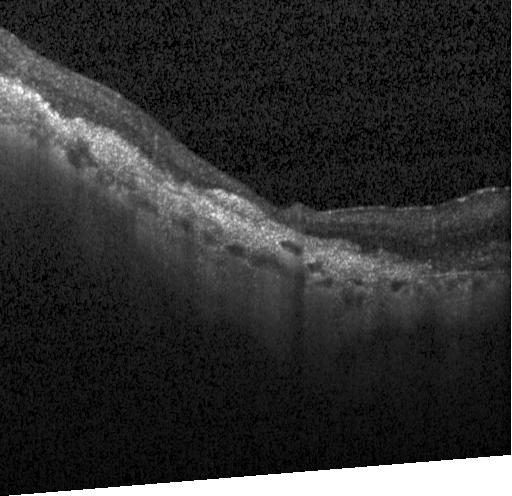
Macular OCT: CNV.